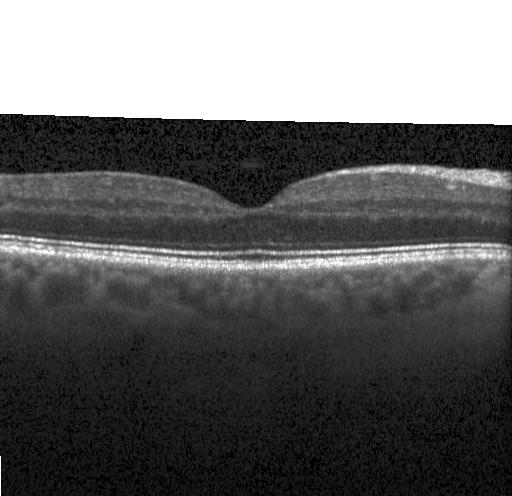
Macular scan · retinal OCT cross-section.
Finding: no CNV, DME, or drusen.